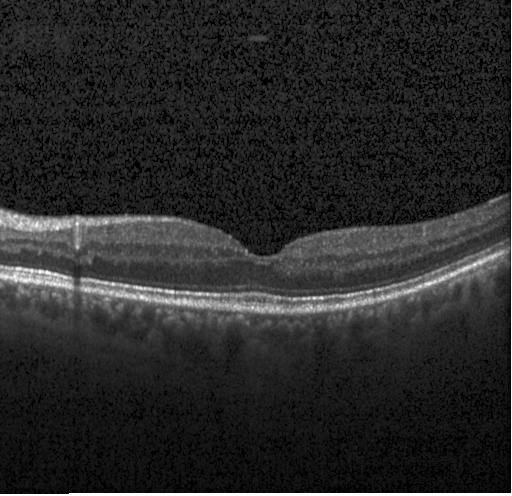

Heidelberg Spectralis. Optical coherence tomography B-scan. Centered on the fovea. Spectral-domain optical coherence tomography
Assessment: neither CNV, DME, nor drusen.